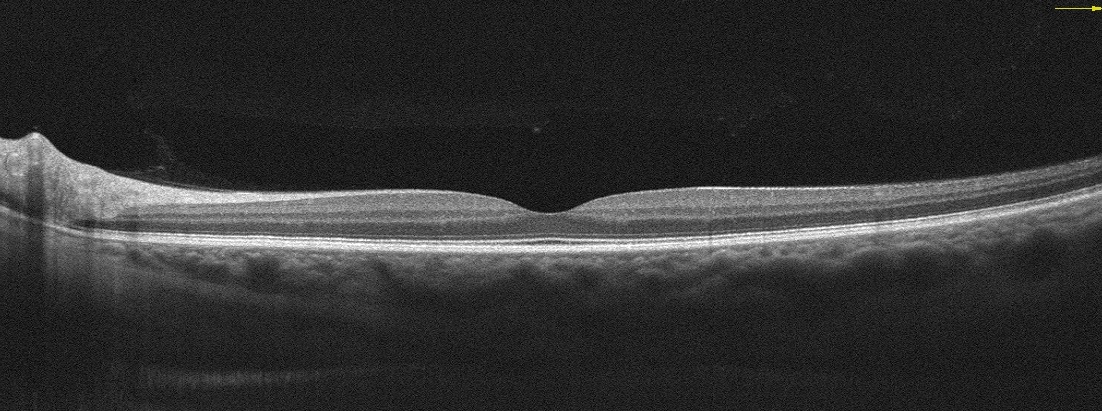

Diagnosis: no evidence of AMD, DME, ERM, RAO, RVO, or VID.